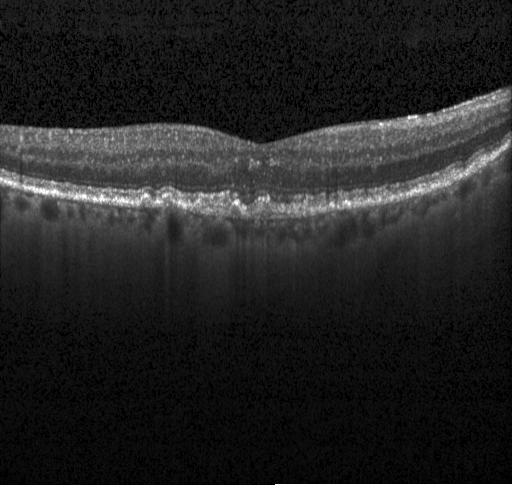

The scan shows multiple drusen.